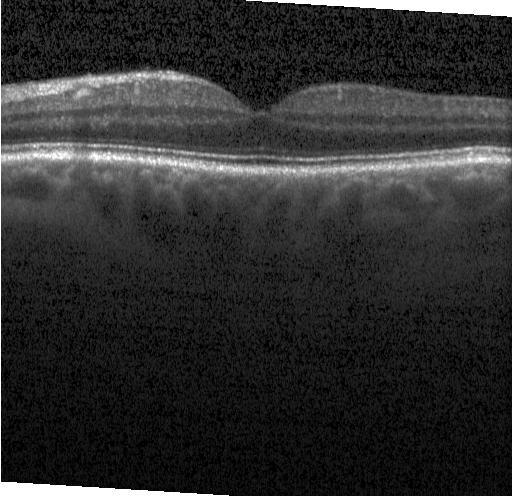
Instrument: Heidelberg Spectralis; macular scan; optical coherence tomography scan; spectral-domain OCT
Impression: no choroidal neovascularization, no diabetic macular edema, and no drusen.